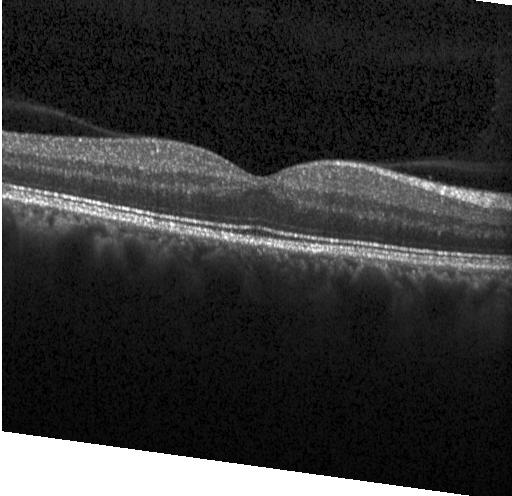
Optical coherence tomography scan · instrument: Heidelberg Spectralis. Diagnosis: no CNV, DME, or drusen.